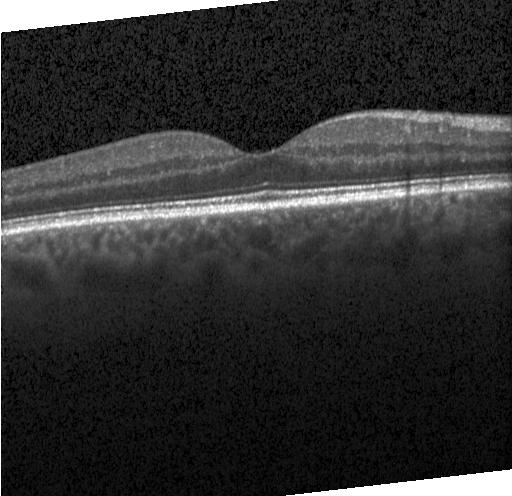

Centered on the fovea. SD-OCT. Optical coherence tomography scan. Acquired on a Heidelberg Spectralis — This B-scan demonstrates no CNV, DME, or drusen.